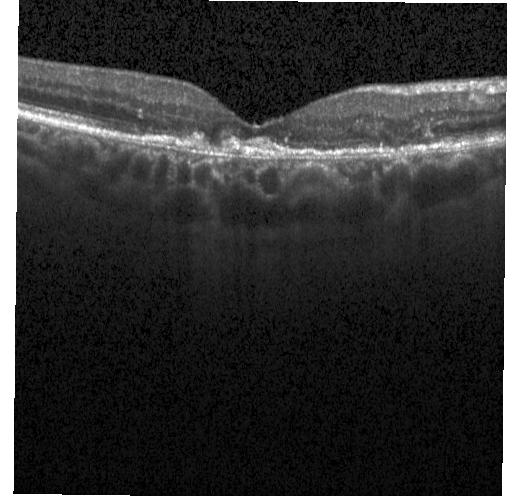 Spectral-domain OCT B-scan: CNV.